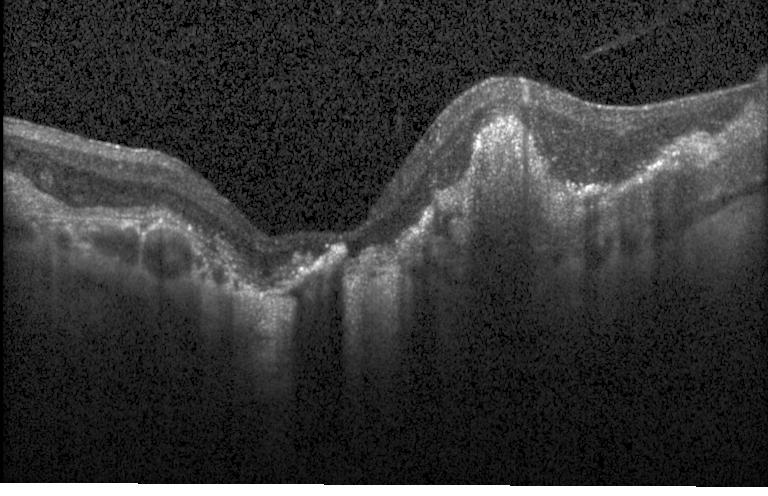 Acquired on a Heidelberg Spectralis; OCT line scan. Diagnosis: CNV.